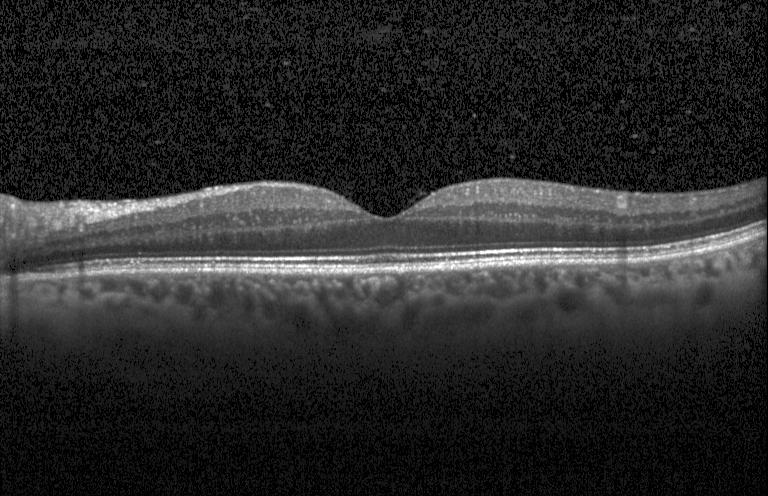 Assessment: no evidence of choroidal neovascularization, diabetic macular edema, or drusen.